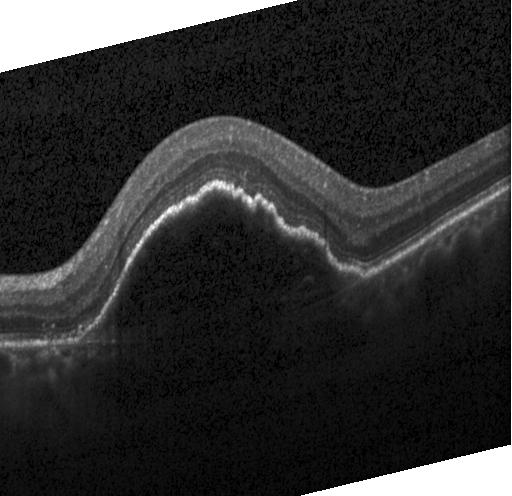

Impression: choroidal neovascularization.